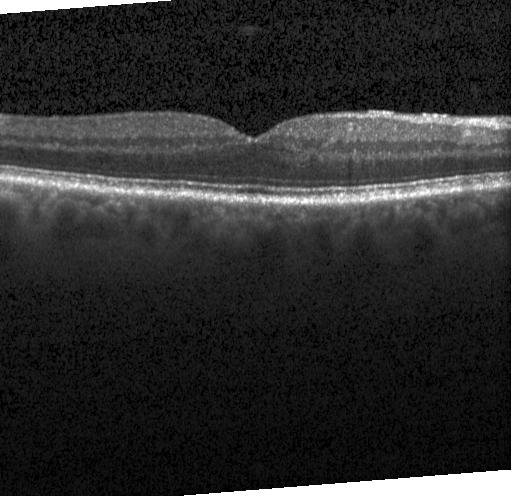 Spectral-domain OCT, retinal OCT cross-section.
Impression: no evidence of choroidal neovascularization, diabetic macular edema, or drusen.